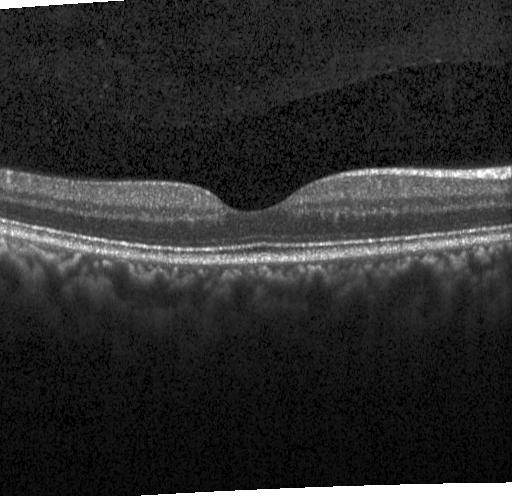 Macular scan; acquired on a Heidelberg Spectralis; spectral-domain optical coherence tomography; optical coherence tomography B-scan — Macular OCT: no choroidal neovascularization, no diabetic macular edema, and no drusen.